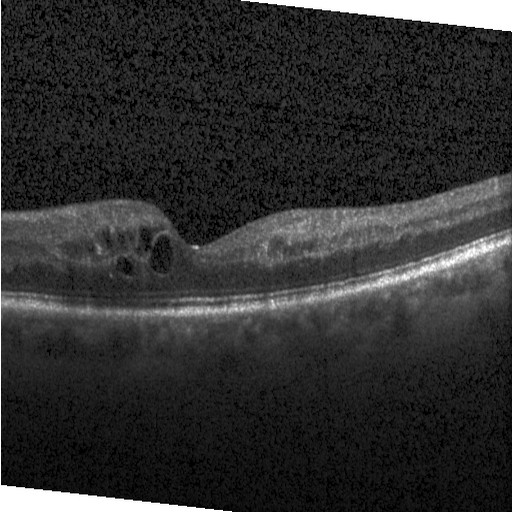
Optical coherence tomography B-scan
OCT finding: diabetic macular edema.